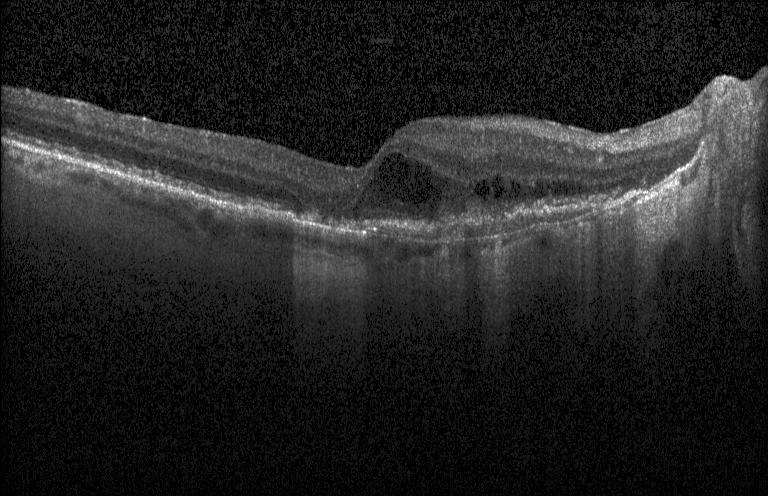
Retinal OCT B-scan · centered on the fovea.
The scan shows a choroidal neovascular membrane.